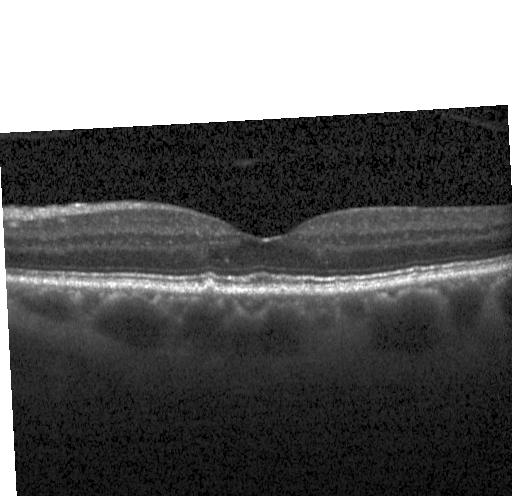

OCT B-scan
Assessment: multiple drusen.